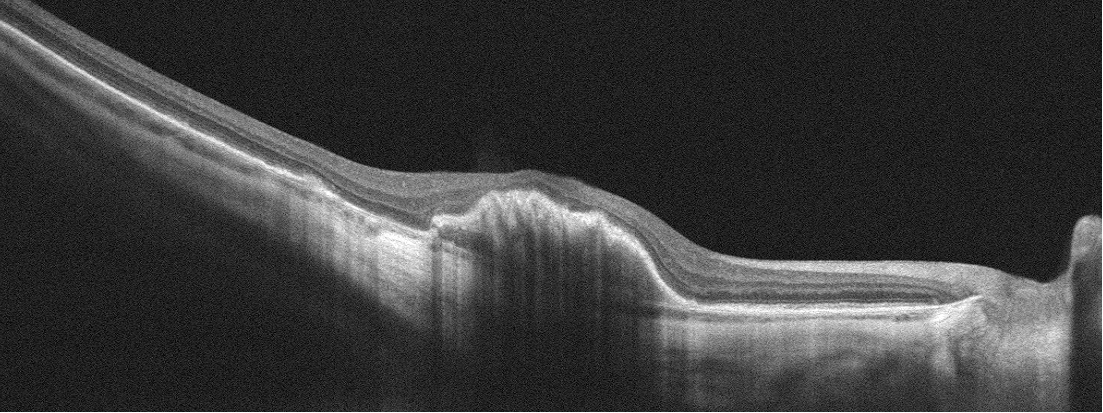
Optovue Avanti RTVue XR; through the macula; optical coherence tomography B-scan — AMD.